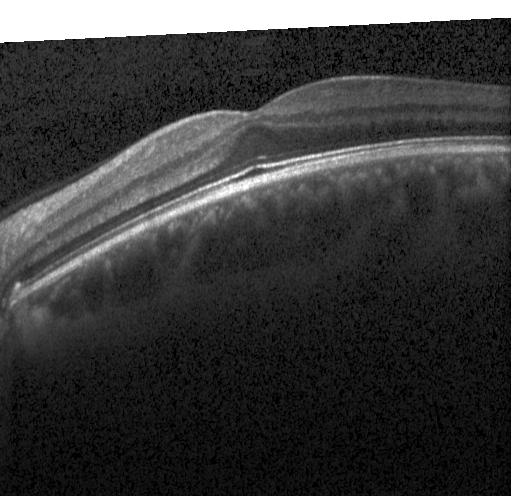

Spectral-domain OCT; retinal OCT cross-section; horizontal scan through the fovea; instrument: Heidelberg Spectralis
Diagnosis: no choroidal neovascularization, diabetic macular edema, or drusen.